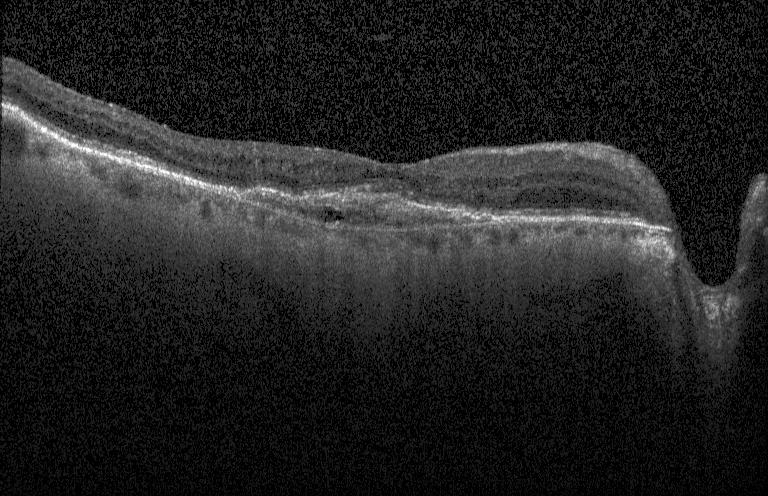
Retinal OCT cross-section, macular scan
Impression: a choroidal neovascular membrane.